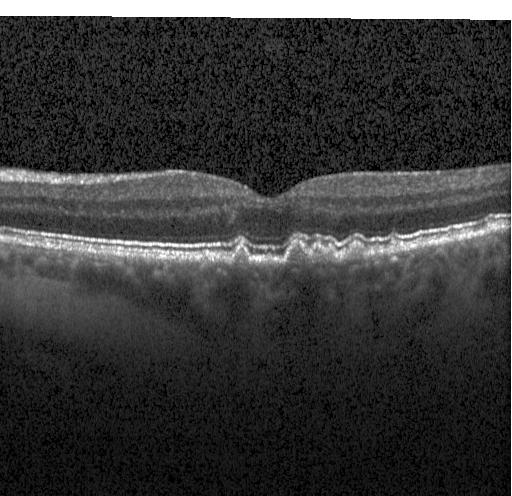 OCT B-scan showing multiple drusen.